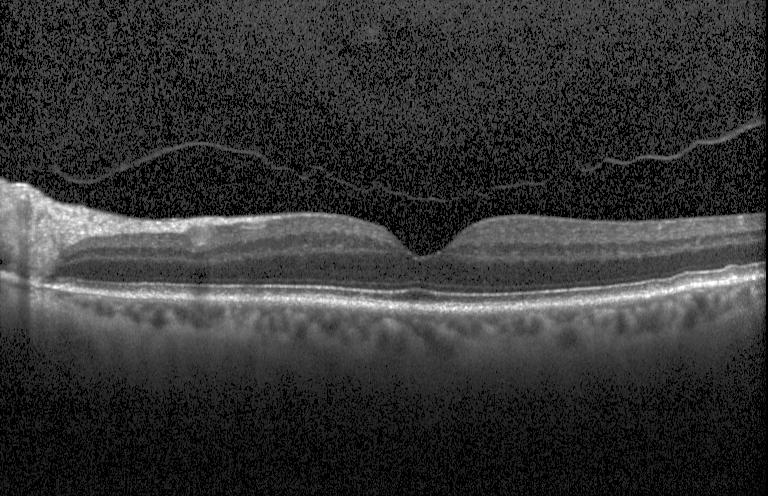 Retinal OCT B-scan.
Finding: no CNV, no DME, and no drusen.